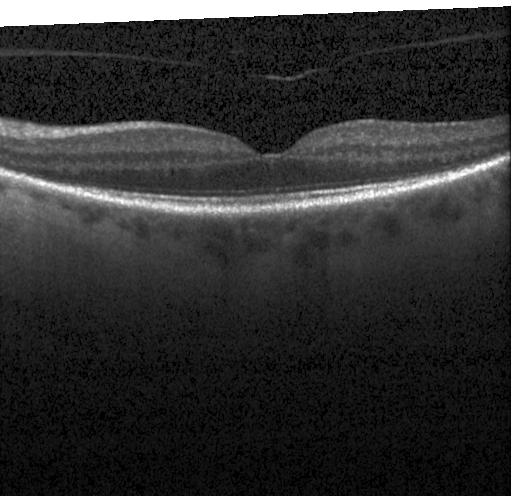
OCT finding: no CNV, no DME, and no drusen.